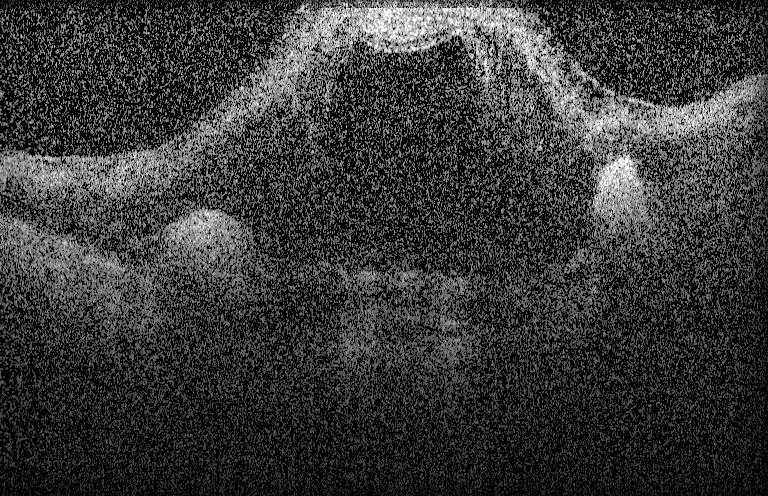

OCT line scan — Impression: a choroidal neovascular membrane.